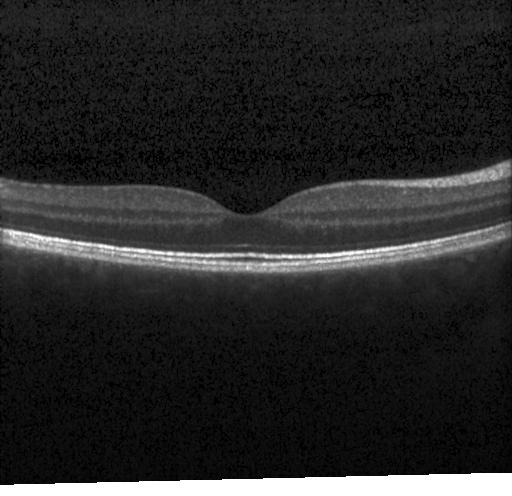

Macular OCT: no choroidal neovascularization, no diabetic macular edema, and no drusen.